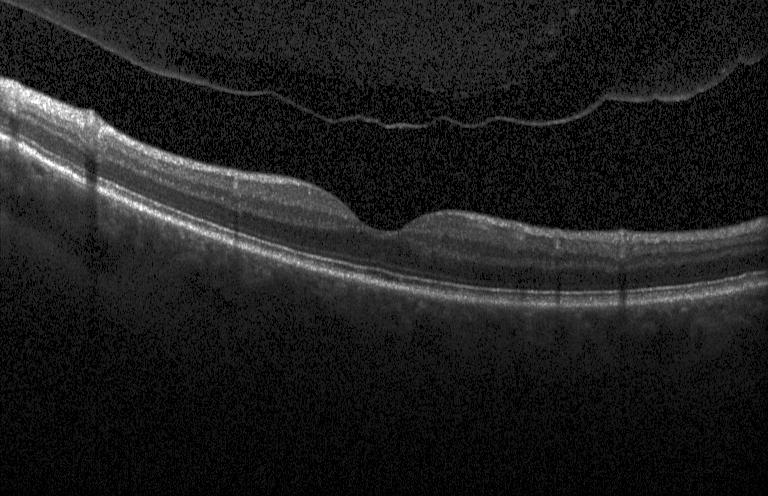 Retinal OCT B-scan. Spectral-domain optical coherence tomography.
No CNV, no DME, and no drusen.